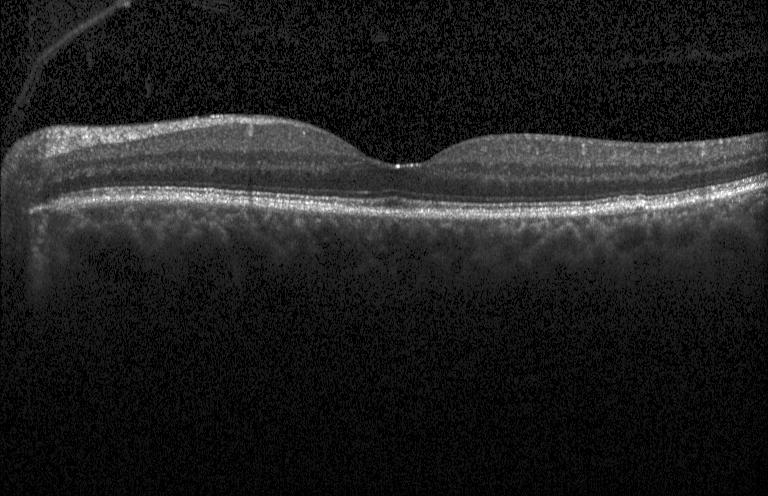 Dx: no CNV, DME, or drusen.